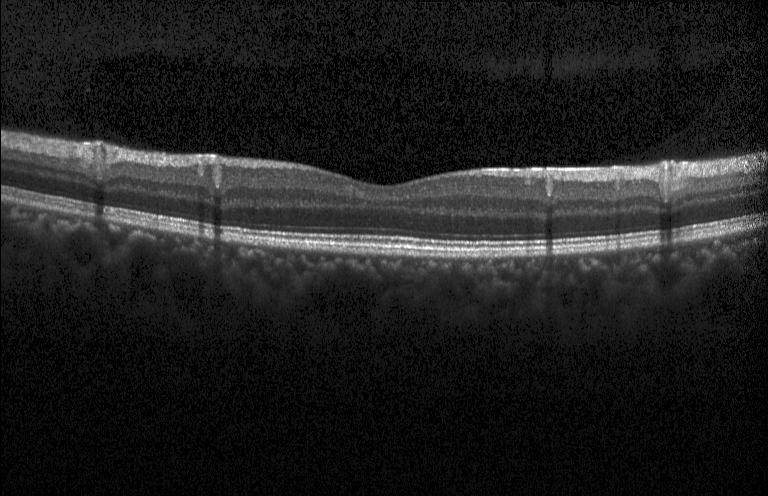 Finding: neither CNV, DME, nor drusen.